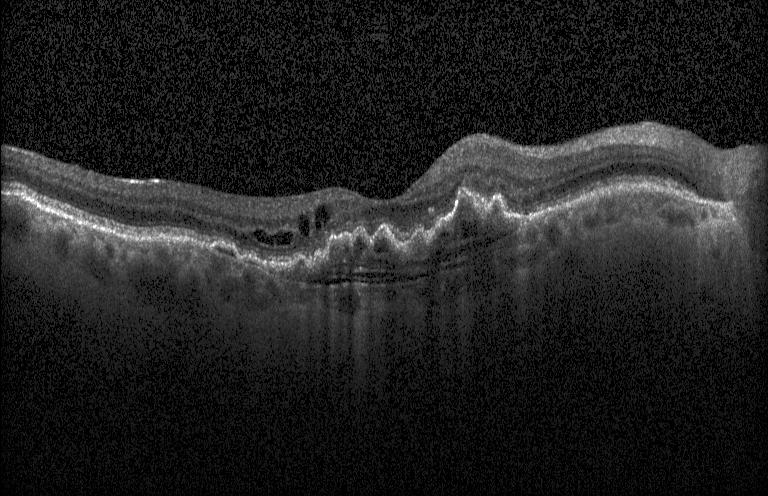
Finding: choroidal neovascularization.